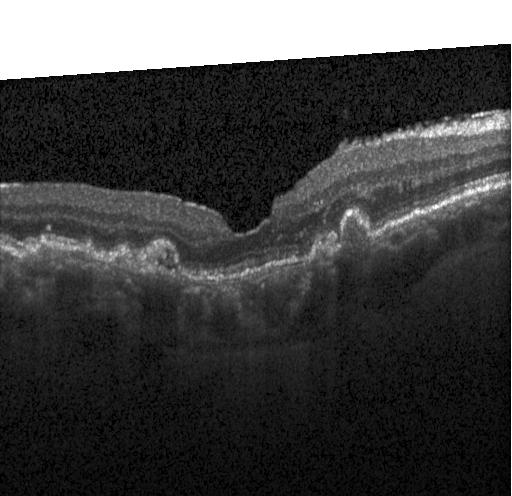
Dx: choroidal neovascularization (CNV).